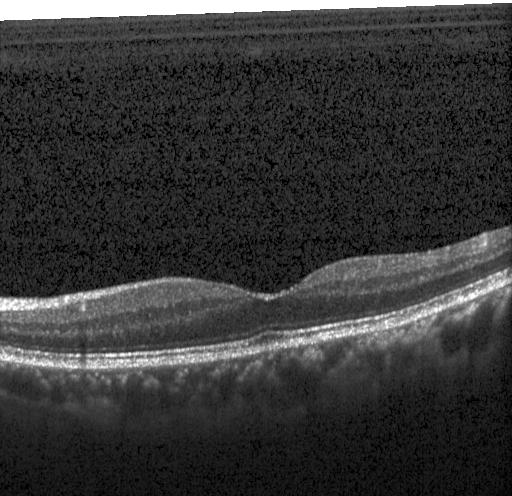
OCT B-scan showing no choroidal neovascularization, diabetic macular edema, or drusen.